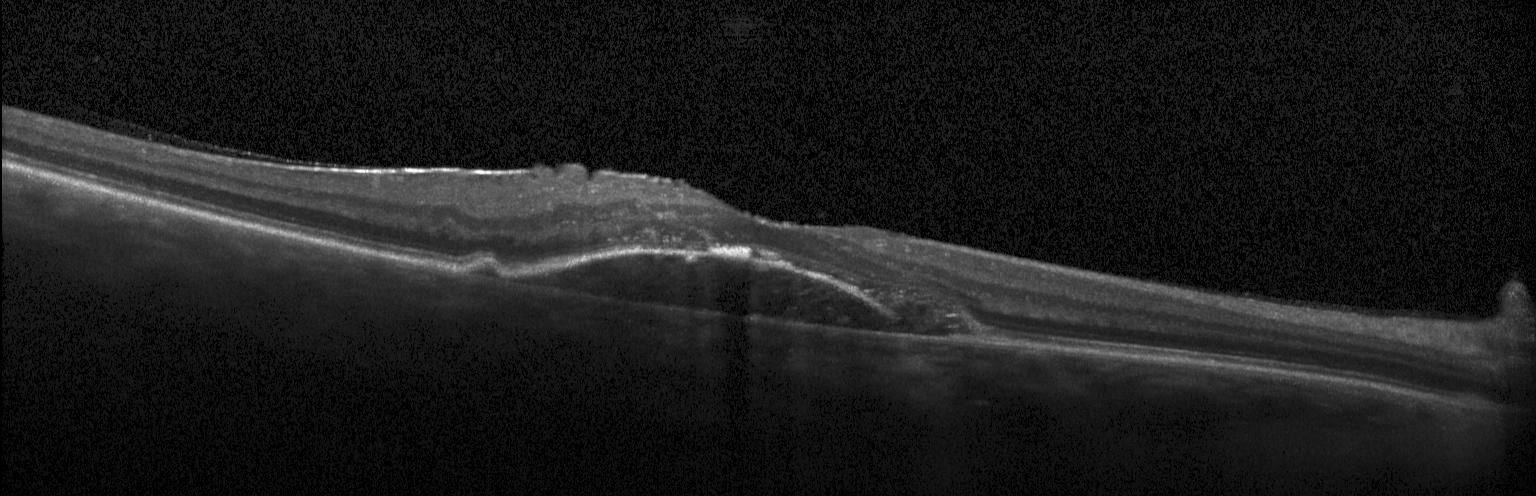
Acquired on a Heidelberg Spectralis. Optical coherence tomography B-scan
Finding: a choroidal neovascular membrane.